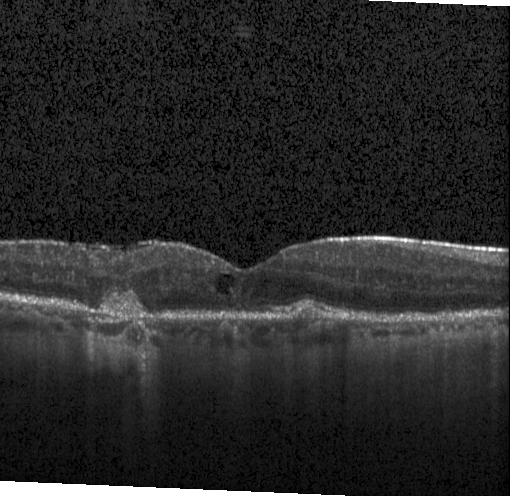 Heidelberg Spectralis. OCT line scan. This B-scan demonstrates CNV.